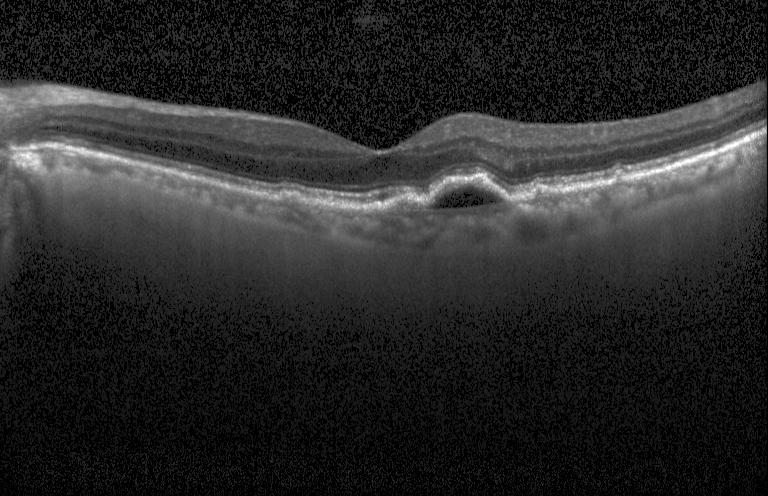
Optical coherence tomography B-scan · SD-OCT.
The scan shows CNV.